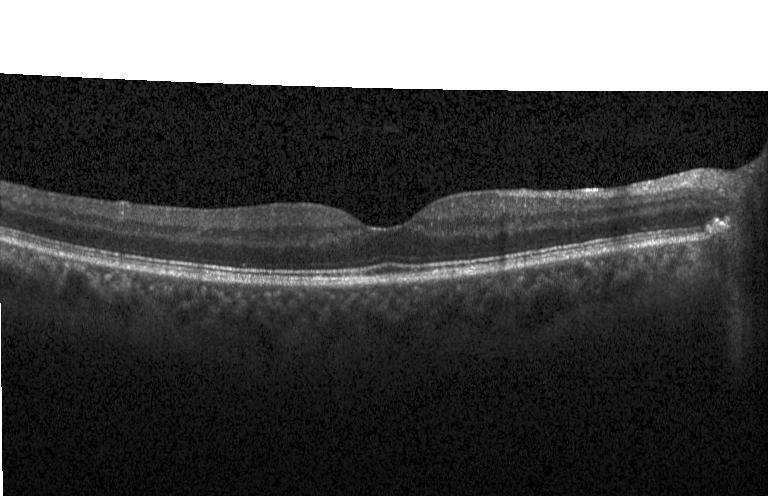 Macular OCT demonstrating no choroidal neovascularization, diabetic macular edema, or drusen.